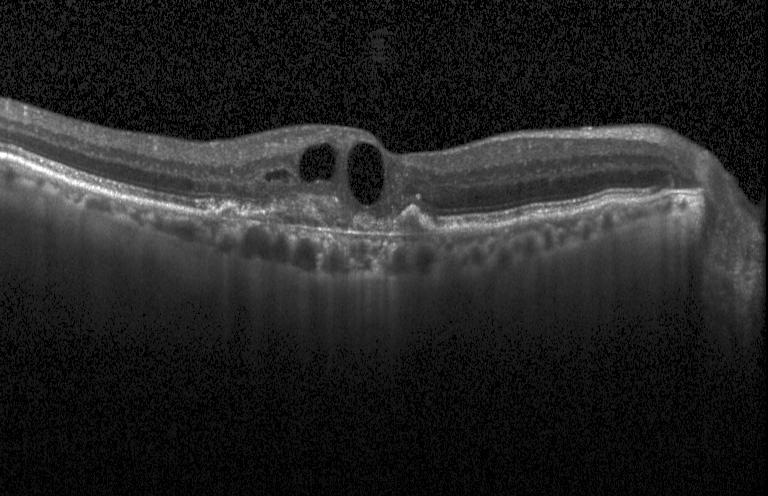

Horizontal scan through the fovea. OCT B-scan. Spectral-domain optical coherence tomography. Acquired on a Heidelberg Spectralis
Dx: a choroidal neovascular membrane.